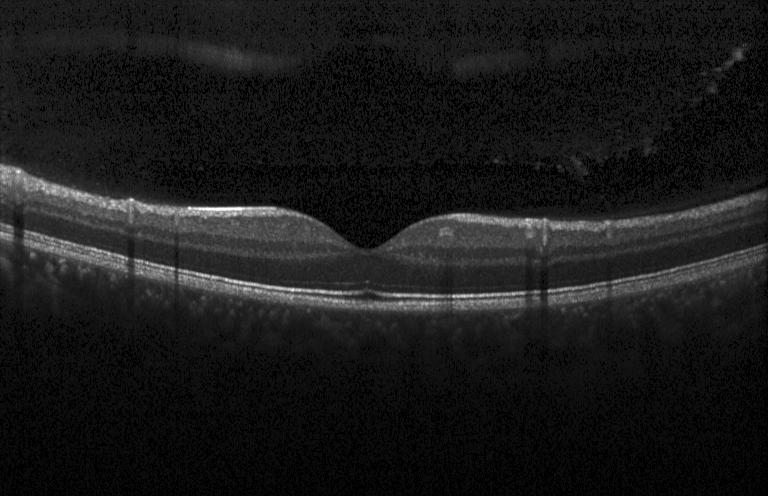 Spectral-domain optical coherence tomography. Fovea-centered. Retinal OCT B-scan. Finding: no CNV, no DME, and no drusen.